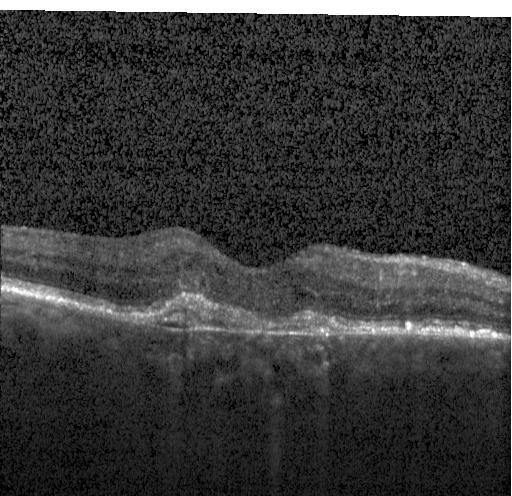
Optical coherence tomography scan. Acquired on a Heidelberg Spectralis — This B-scan demonstrates CNV.